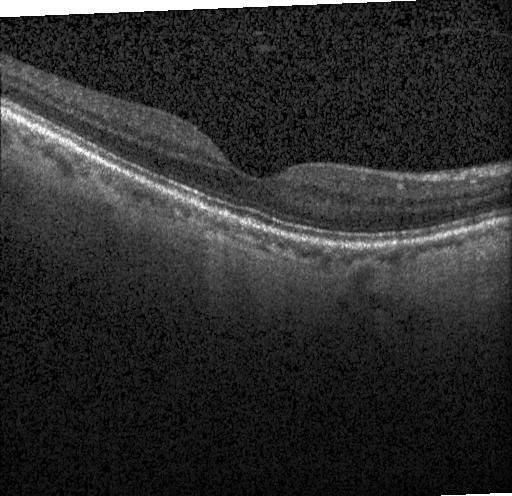

Optical coherence tomography scan; SD-OCT; macular scan; Heidelberg Spectralis. Impression: no evidence of choroidal neovascularization, diabetic macular edema, or drusen.